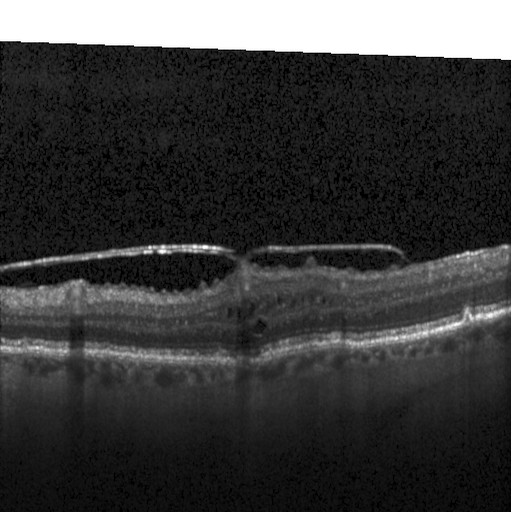 Macular scan. Retinal OCT B-scan. Spectral-domain optical coherence tomography
Diagnosis: diabetic macular edema.